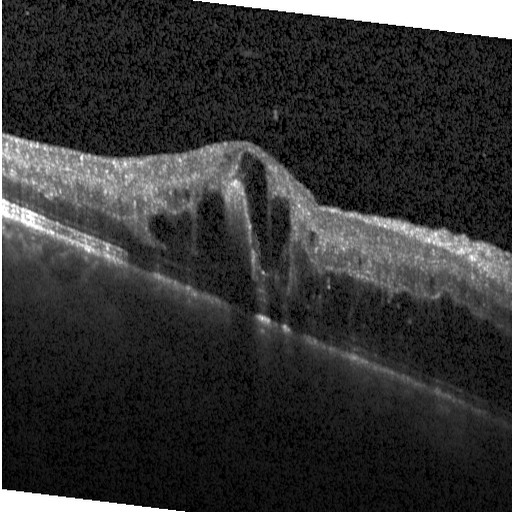
OCT B-scan · SD-OCT — OCT finding: diabetic macular edema.